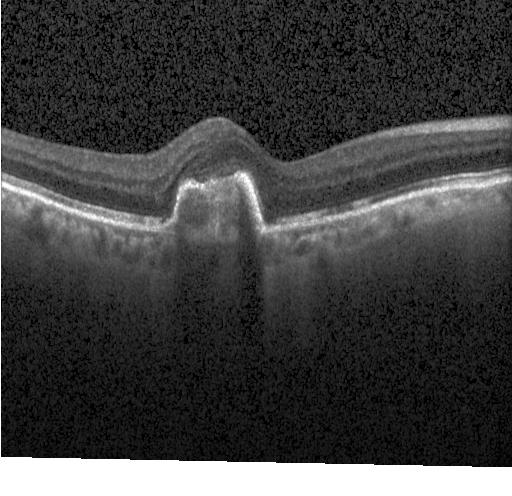

Optical coherence tomography scan. Macular OCT: a choroidal neovascular membrane.